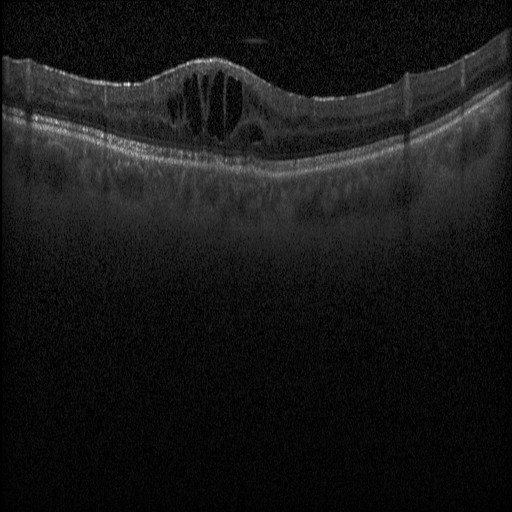 Retinal OCT B-scan. Assessment: diabetic macular edema (DME).